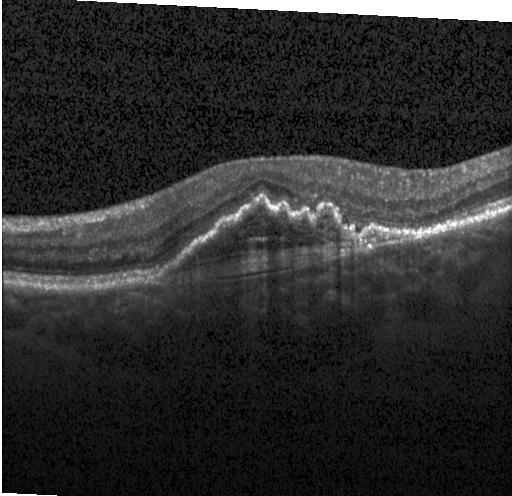

OCT line scan — A choroidal neovascular membrane.